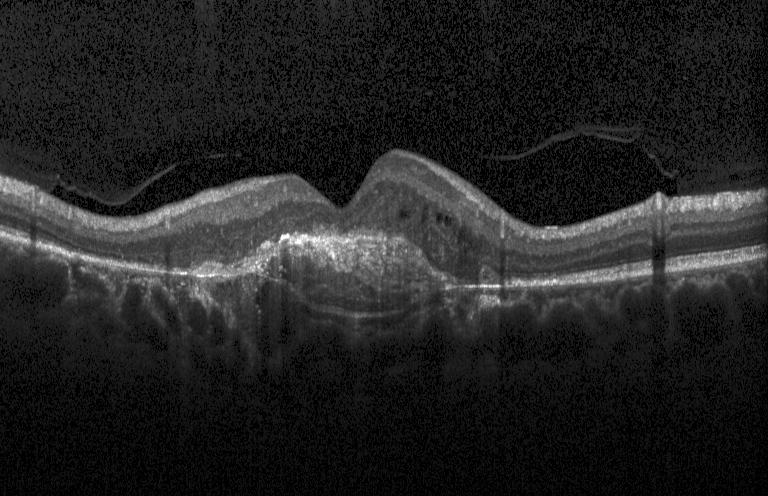 Spectral-domain optical coherence tomography; retinal OCT B-scan
Diagnosis: a choroidal neovascular membrane.